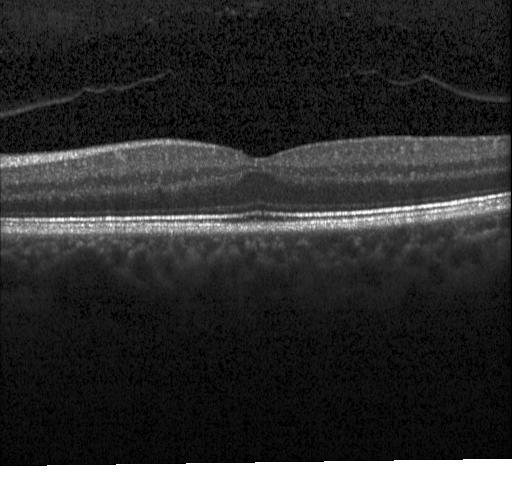 Assessment: no choroidal neovascularization, diabetic macular edema, or drusen.